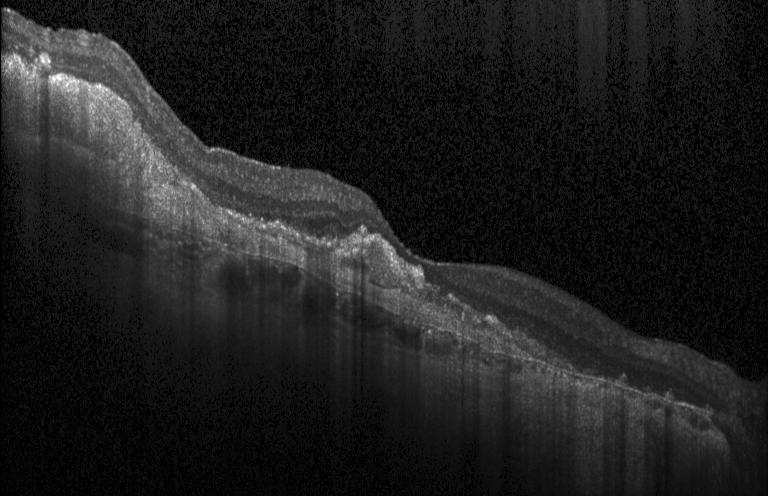

SD-OCT. Retinal OCT cross-section.
The scan shows choroidal neovascularization.